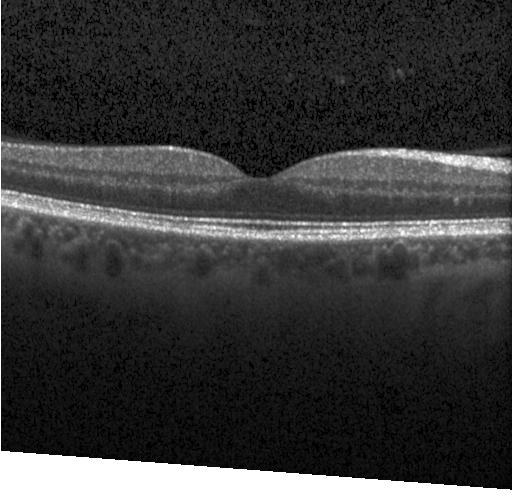

Diagnosis: no evidence of choroidal neovascularization, diabetic macular edema, or drusen.